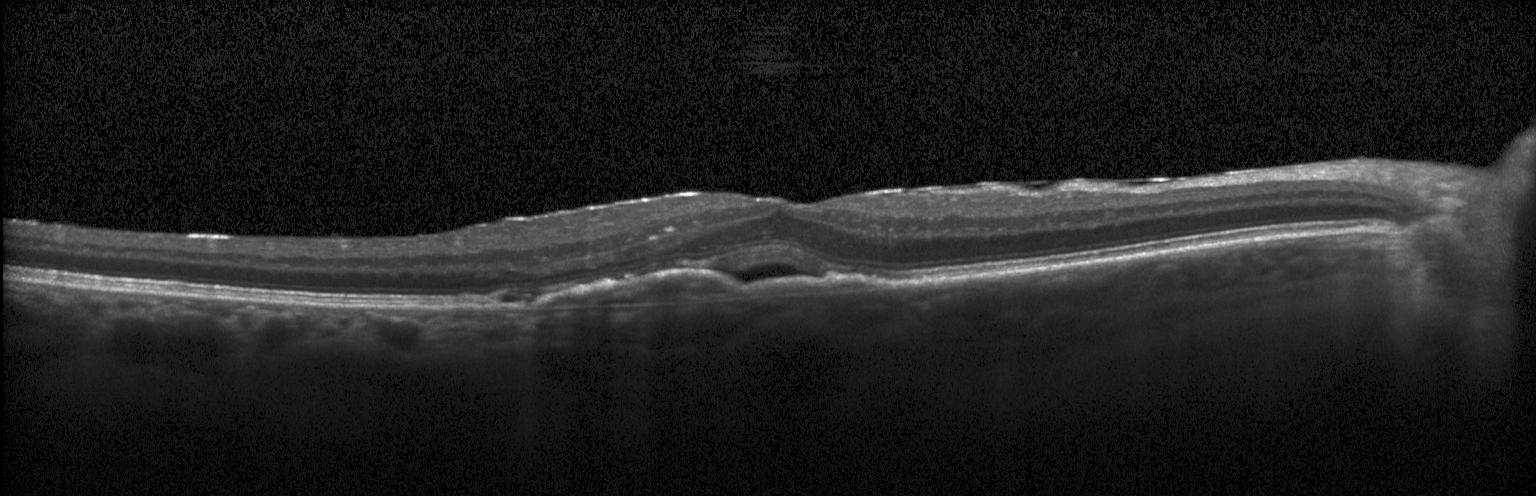 Macular OCT: CNV.